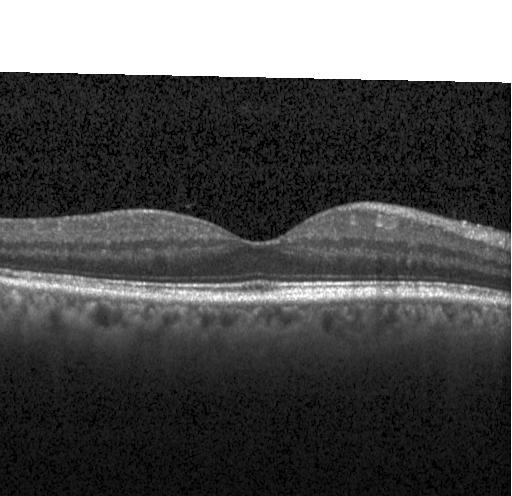
Instrument: Heidelberg Spectralis · spectral-domain optical coherence tomography · optical coherence tomography scan. No choroidal neovascularization, diabetic macular edema, or drusen.